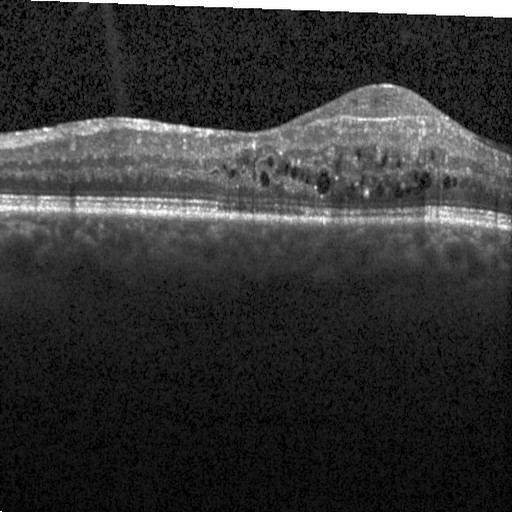

Spectral-domain OCT B-scan: diabetic macular edema.